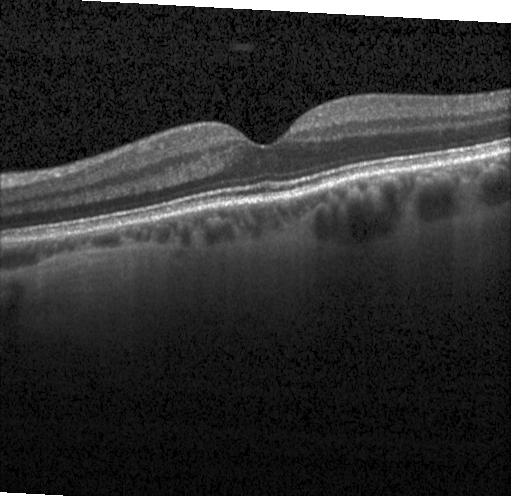 Macular OCT: no choroidal neovascularization, no diabetic macular edema, and no drusen.